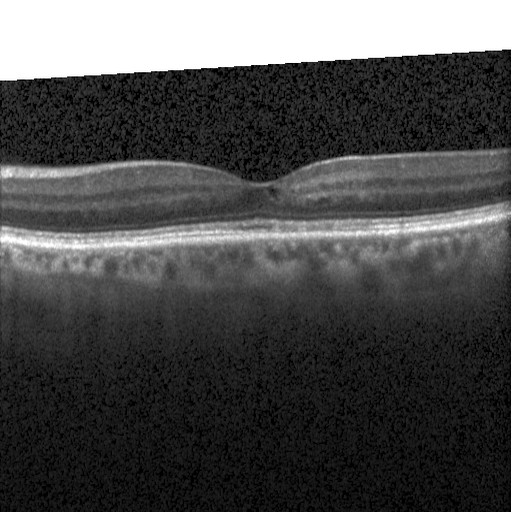 Dx: diabetic macular edema (DME).